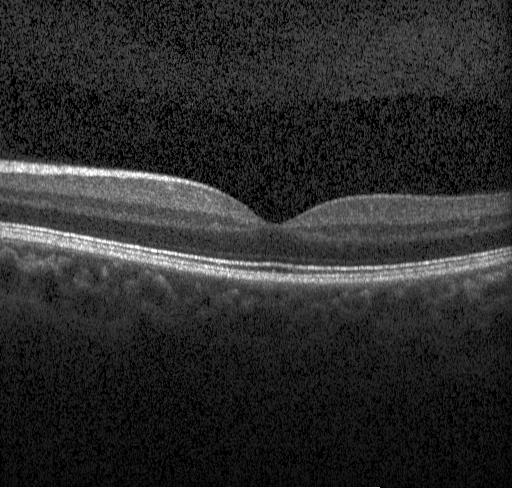 OCT line scan; spectral-domain OCT; fovea-centered — The scan shows no choroidal neovascularization, no diabetic macular edema, and no drusen.